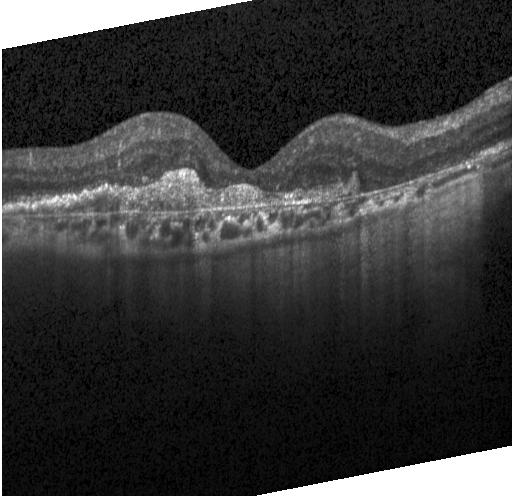

A choroidal neovascular membrane.